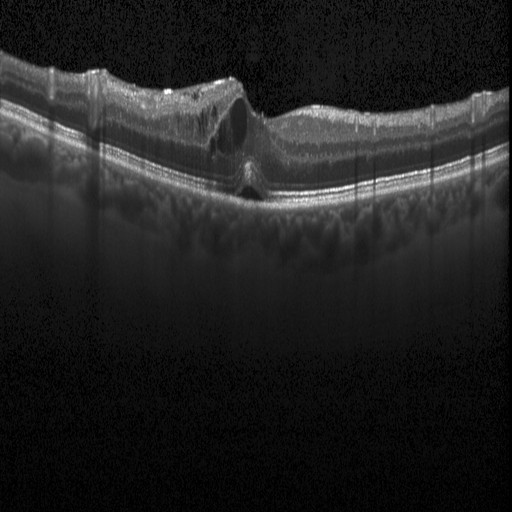
OCT line scan. Finding: DME.